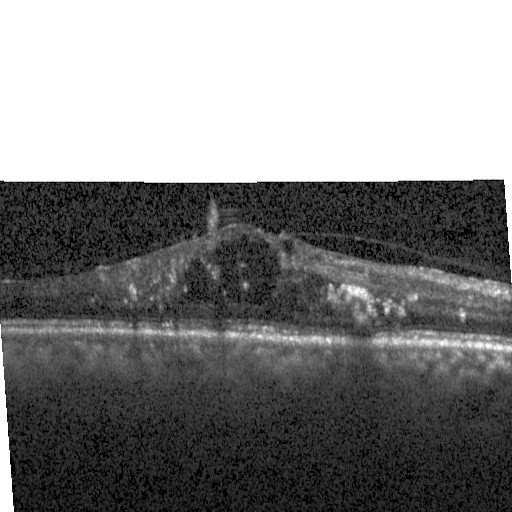

OCT scan showing diabetic macular edema (DME).